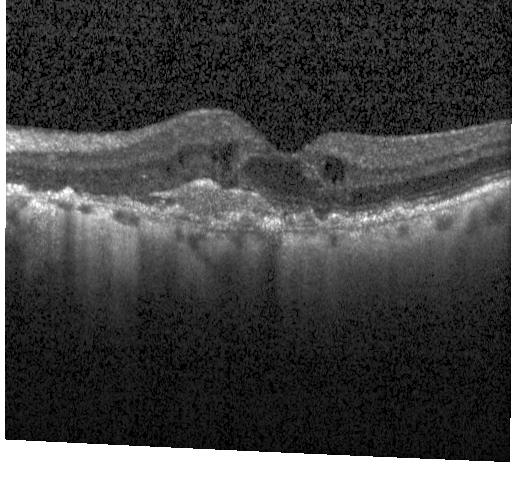 Optical coherence tomography scan; spectral-domain OCT. This B-scan demonstrates a choroidal neovascular membrane.